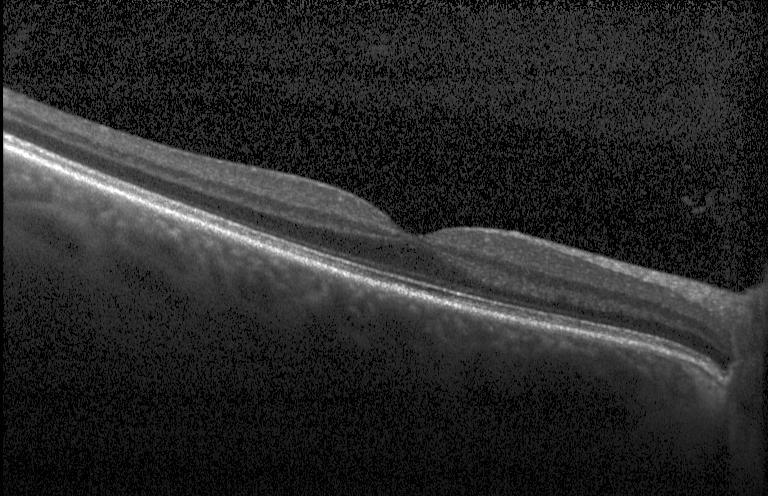
OCT finding: no choroidal neovascularization, diabetic macular edema, or drusen.